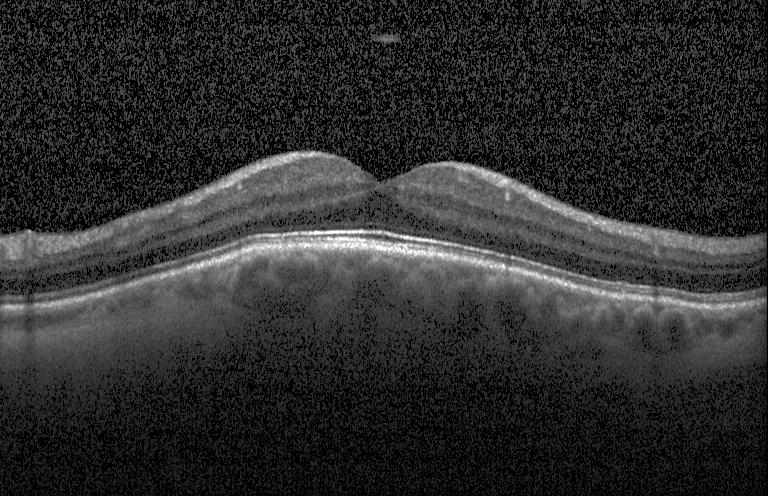
Instrument: Heidelberg Spectralis. Optical coherence tomography B-scan.
Impression: neither choroidal neovascularization, diabetic macular edema, nor drusen.